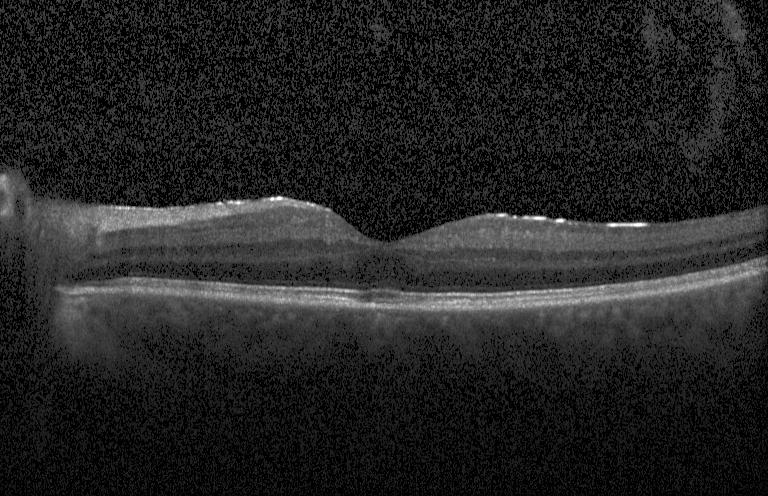 Fovea-centered · instrument: Heidelberg Spectralis · retinal OCT B-scan. Neither choroidal neovascularization, diabetic macular edema, nor drusen.